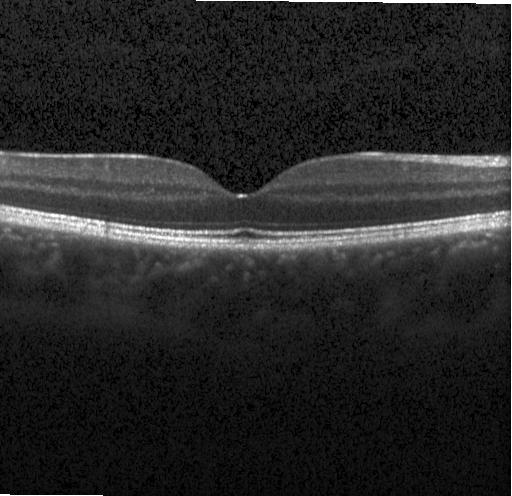
Spectral-domain OCT · OCT line scan · Heidelberg Spectralis OCT system · fovea-centered. OCT finding: no evidence of choroidal neovascularization, diabetic macular edema, or drusen.